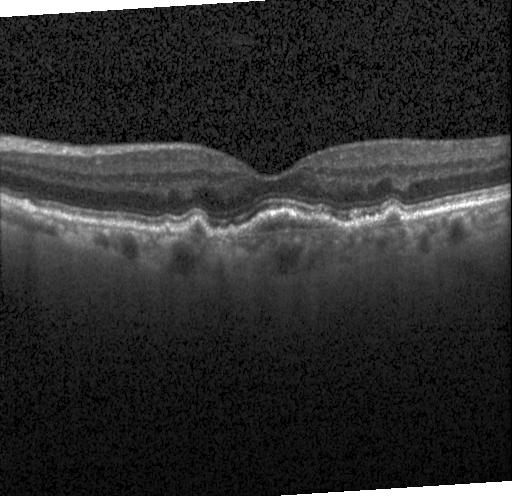

Finding: a choroidal neovascular membrane.